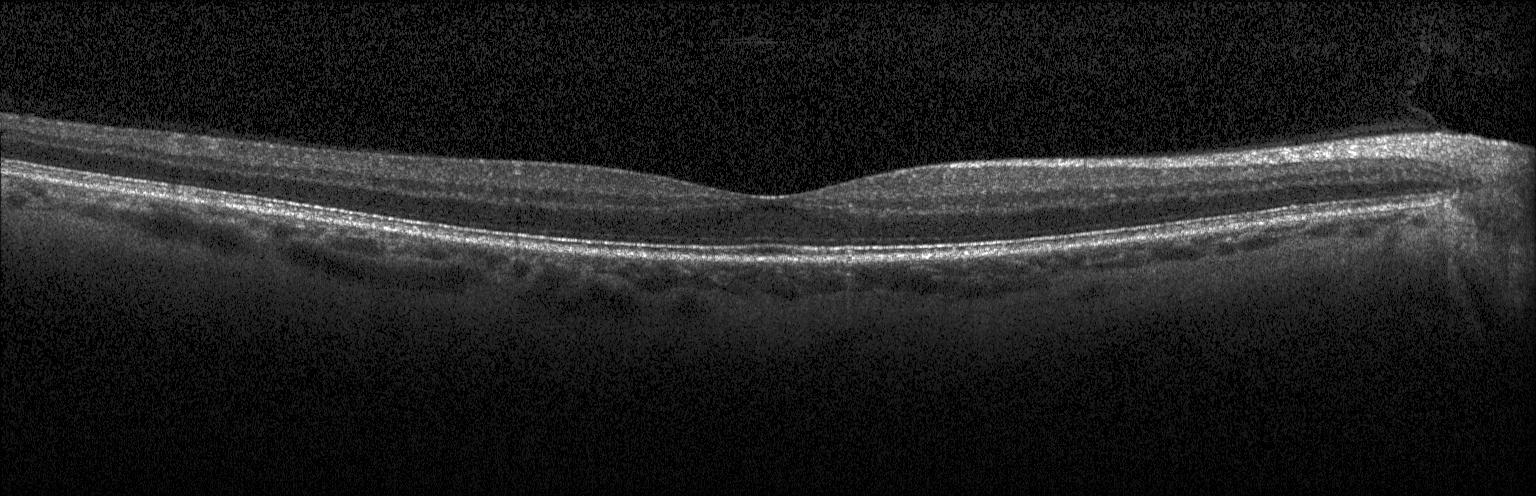
This B-scan demonstrates no evidence of choroidal neovascularization, diabetic macular edema, or drusen.